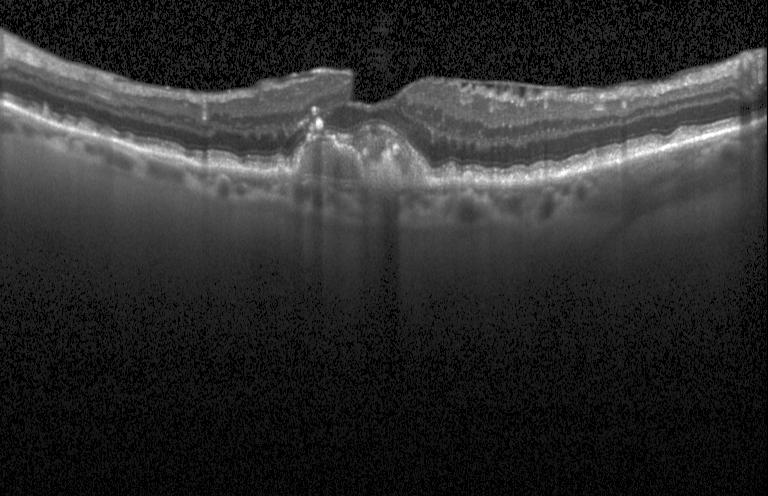
SD-OCT; instrument: Heidelberg Spectralis; optical coherence tomography scan.
OCT finding: choroidal neovascularization (CNV).